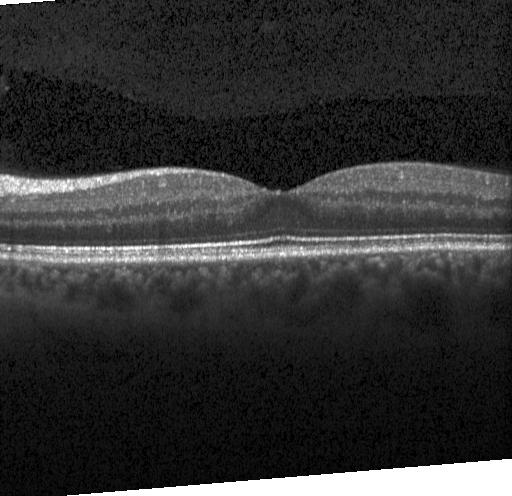 OCT B-scan showing no choroidal neovascularization, diabetic macular edema, or drusen.